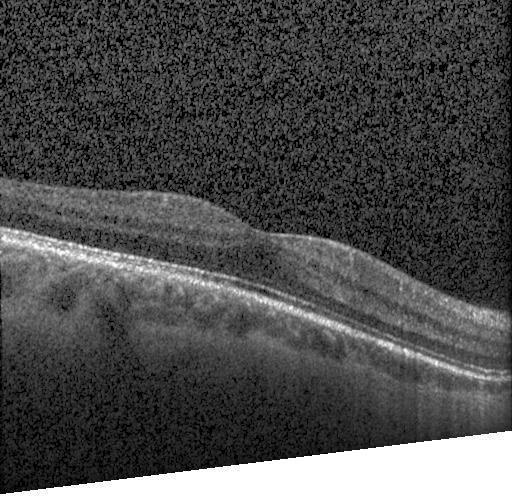 Macular OCT demonstrating neither CNV, DME, nor drusen.